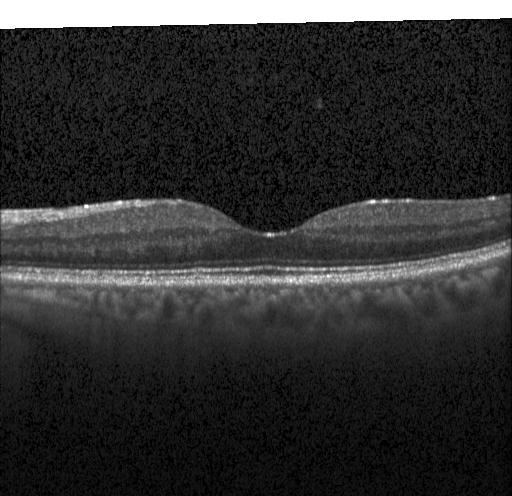

OCT B-scan showing no choroidal neovascularization, diabetic macular edema, or drusen.